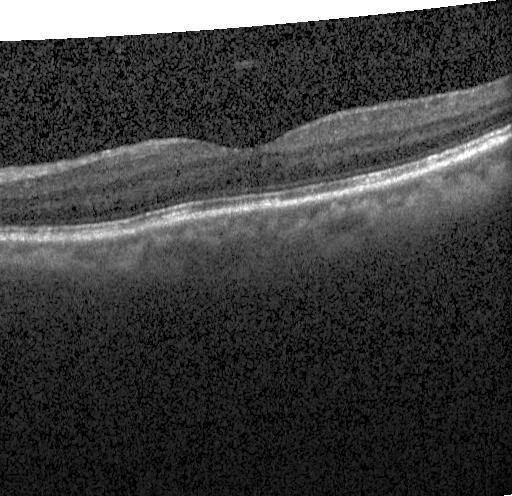
Retinal OCT B-scan. Impression: no evidence of CNV, DME, or drusen.